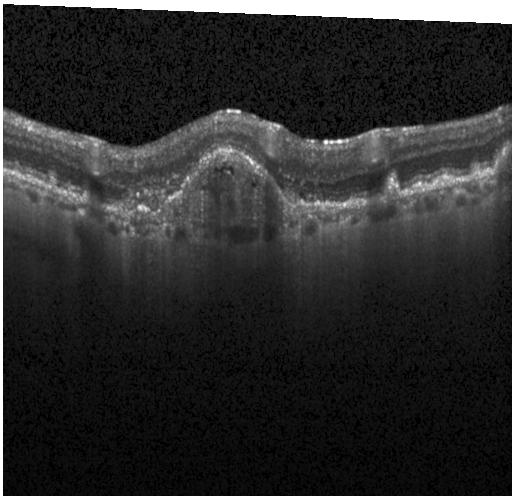

Retinal OCT B-scan, spectral-domain optical coherence tomography — Dx: CNV.